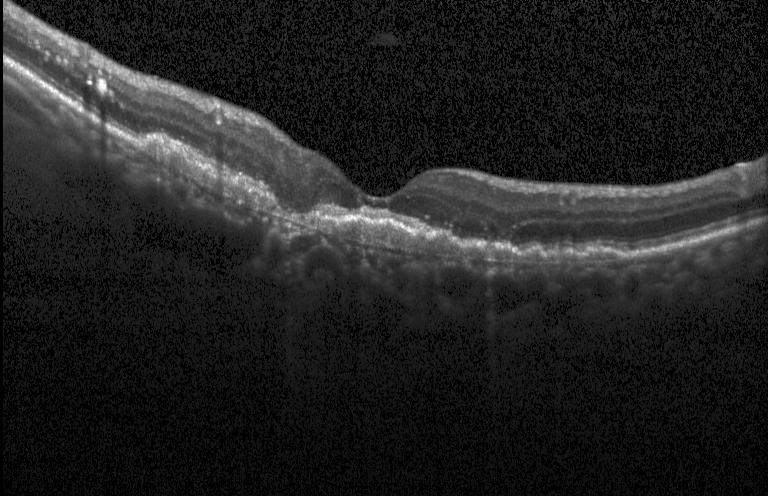 OCT finding: choroidal neovascularization.